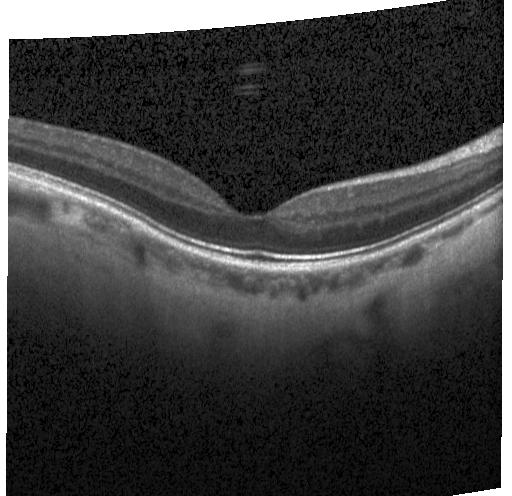

OCT line scan
Diagnosis: neither CNV, DME, nor drusen.